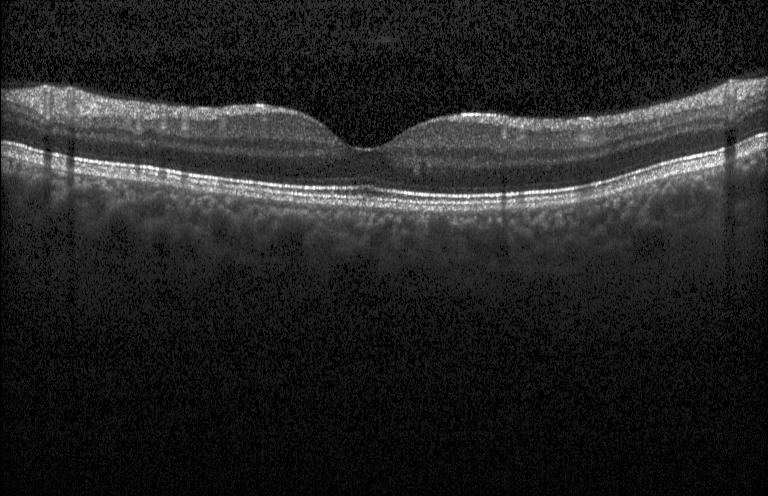

The scan shows no choroidal neovascularization, diabetic macular edema, or drusen.